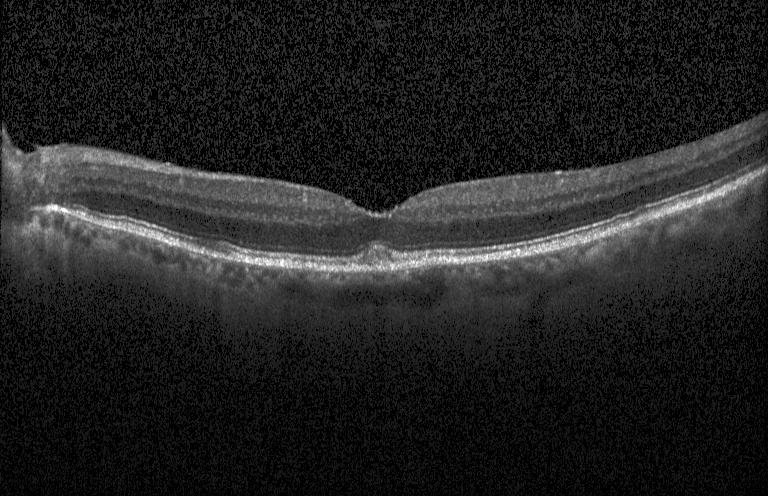 Horizontal scan through the fovea; optical coherence tomography scan. The scan shows multiple drusen.